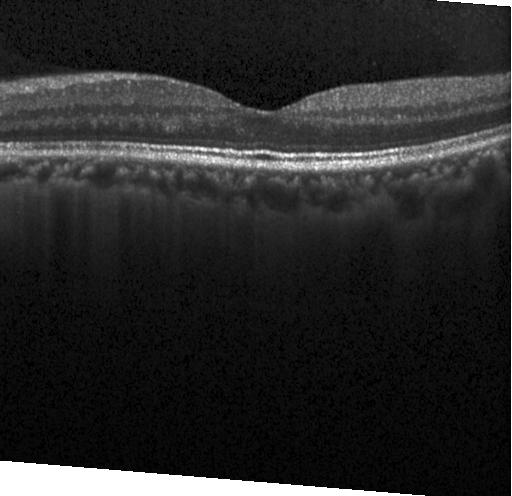 Spectral-domain optical coherence tomography, retinal OCT cross-section, acquired on a Heidelberg Spectralis, through the macula
Finding: no choroidal neovascularization, diabetic macular edema, or drusen.